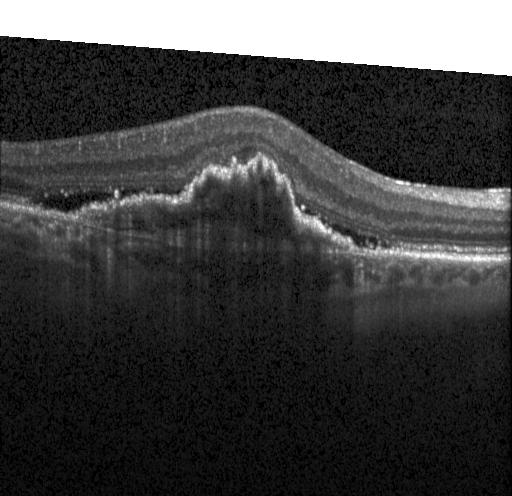
Acquired on a Heidelberg Spectralis · SD-OCT · horizontal scan through the fovea · optical coherence tomography B-scan. Choroidal neovascularization (CNV).